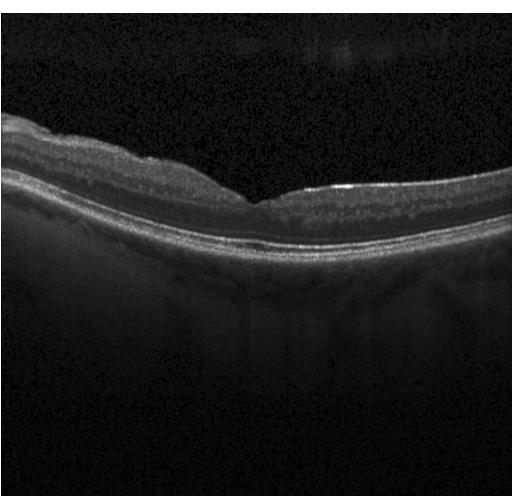

Dx: neither choroidal neovascularization, diabetic macular edema, nor drusen.